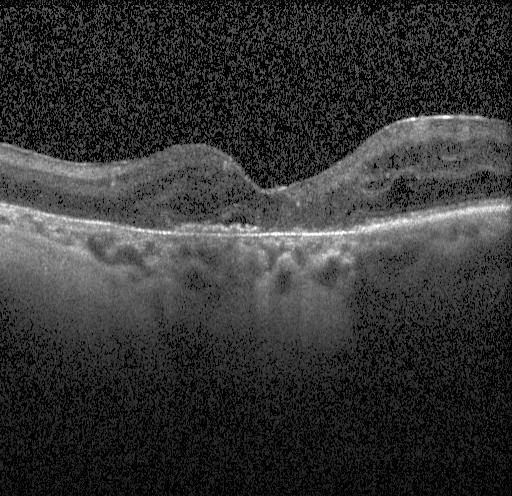 OCT finding: choroidal neovascularization (CNV).